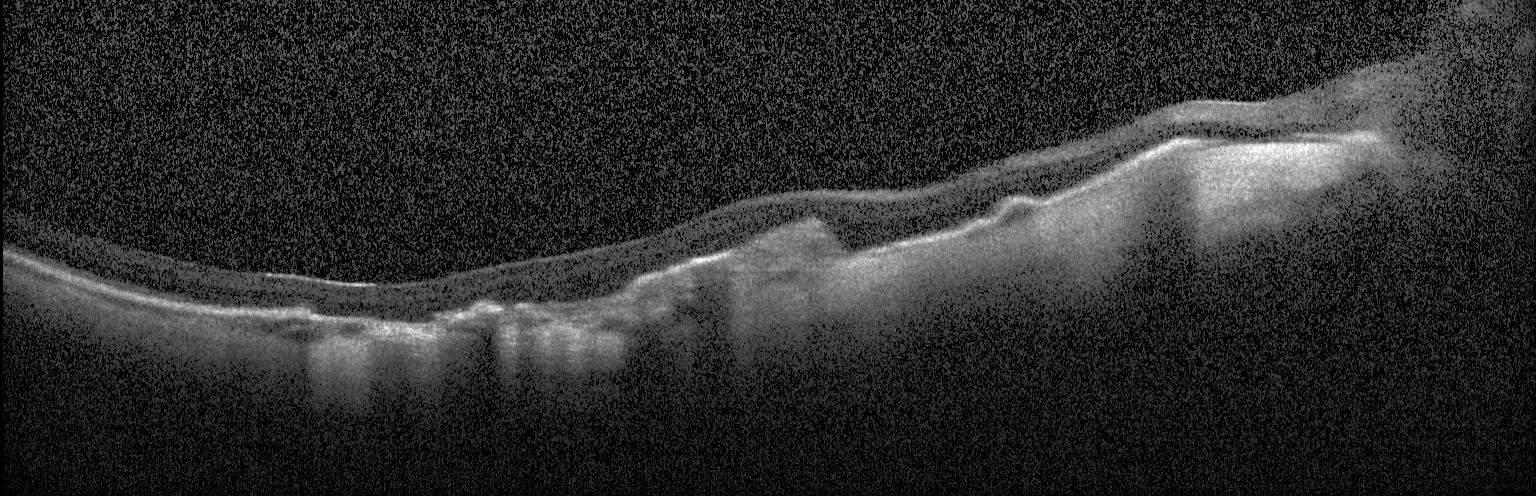
OCT scan showing a choroidal neovascular membrane.